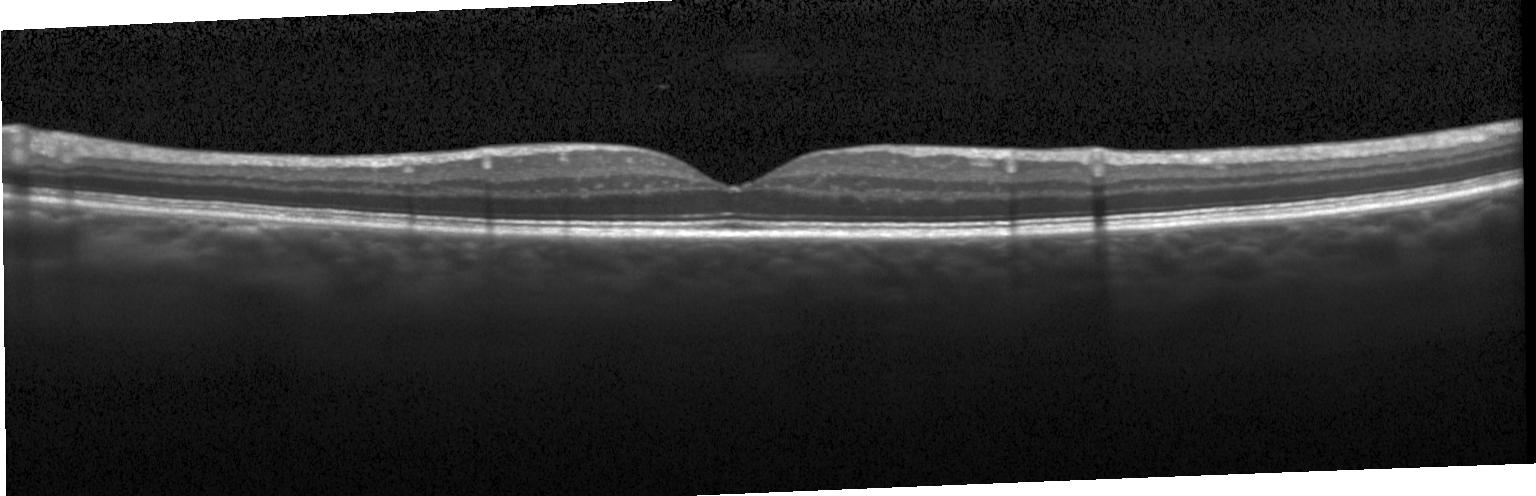
Impression: no choroidal neovascularization, no diabetic macular edema, and no drusen.